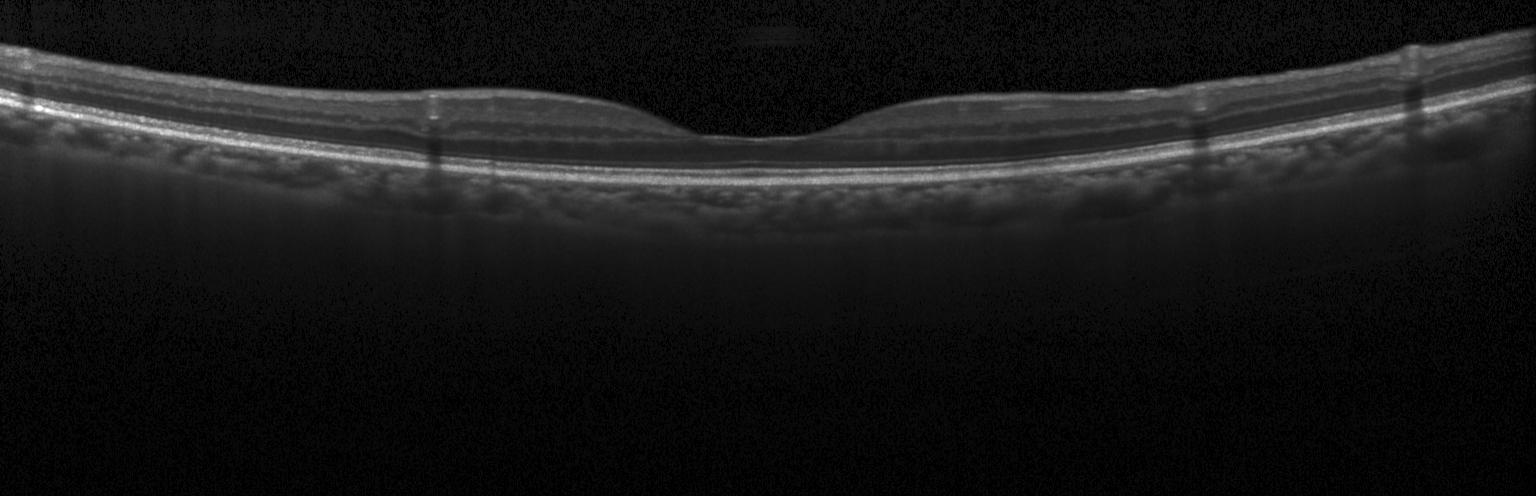 Fovea-centered · OCT line scan · spectral-domain optical coherence tomography. The scan shows no choroidal neovascularization, diabetic macular edema, or drusen.